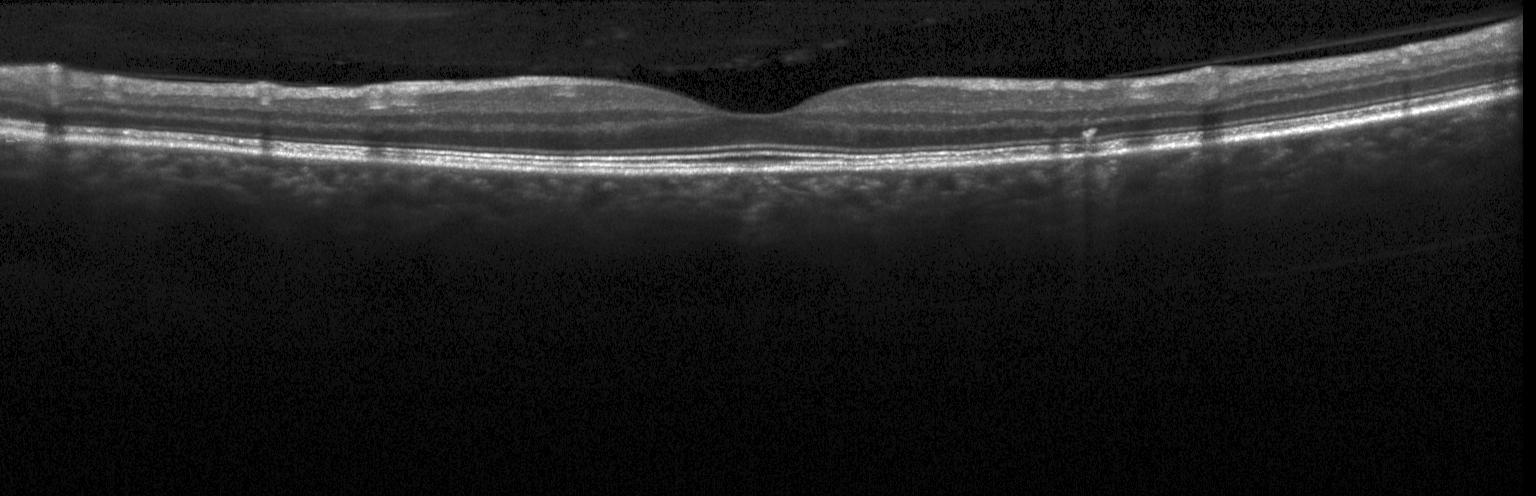

Spectral-domain OCT; optical coherence tomography B-scan — The scan shows no evidence of CNV, DME, or drusen.